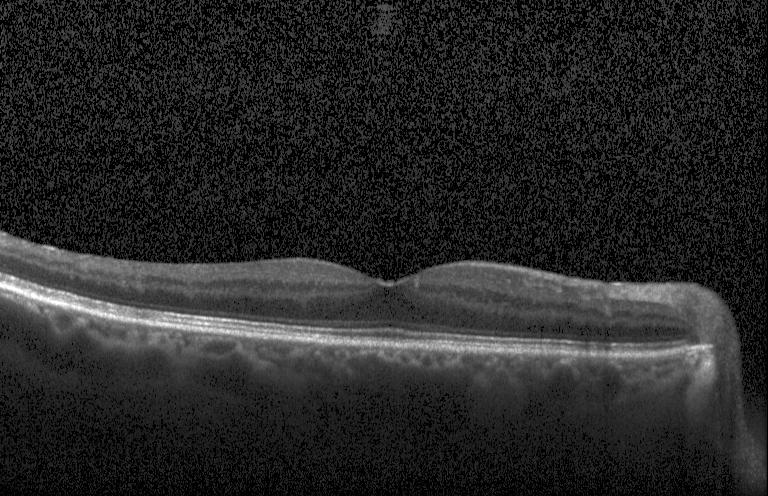 Retinal OCT cross-section, centered on the fovea, acquired on a Heidelberg Spectralis
Neither choroidal neovascularization, diabetic macular edema, nor drusen.